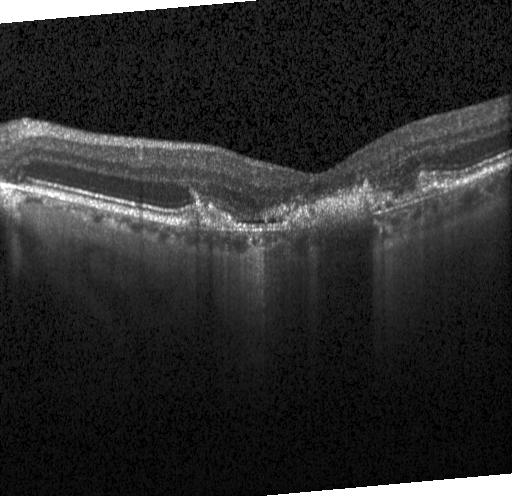
Finding: a choroidal neovascular membrane.